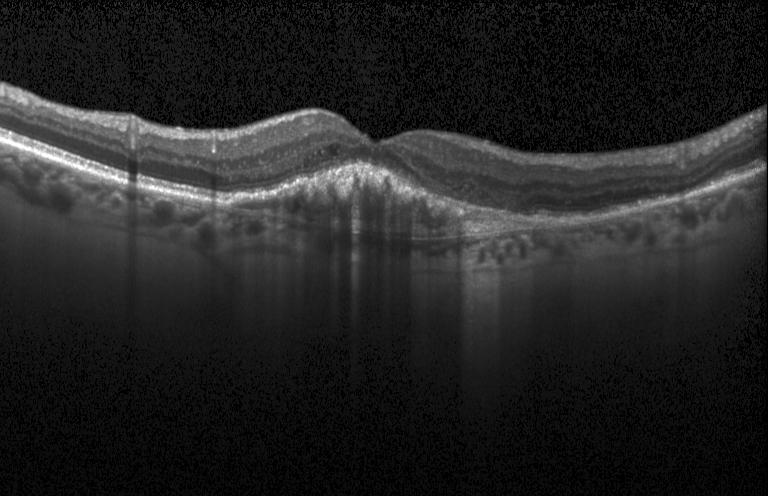

Macular OCT: choroidal neovascularization (CNV).